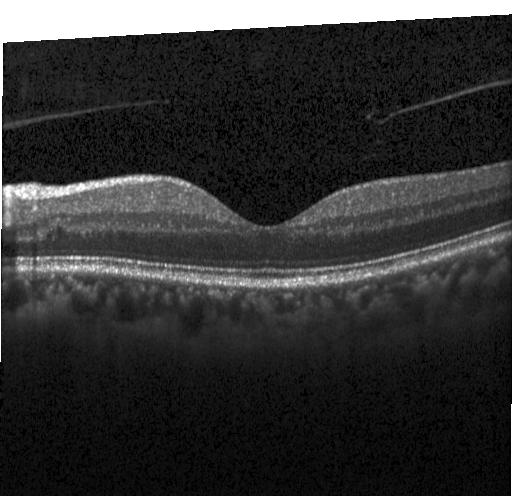
Optical coherence tomography scan · spectral-domain optical coherence tomography · Heidelberg Spectralis OCT system
The scan shows no choroidal neovascularization, no diabetic macular edema, and no drusen.